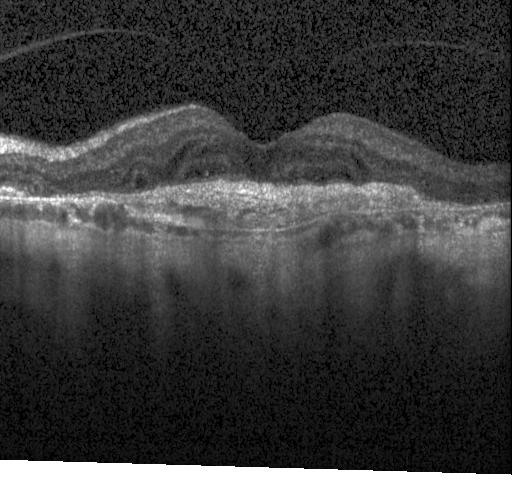

Optical coherence tomography B-scan. Spectral-domain optical coherence tomography. Macular scan. Heidelberg Spectralis
Dx: choroidal neovascularization (CNV).